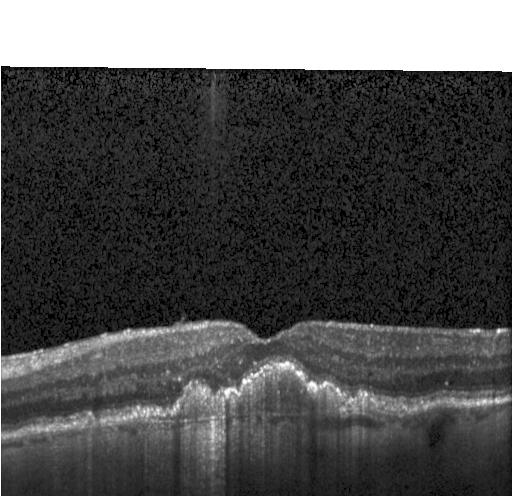 Macular scan. Spectral-domain OCT. OCT line scan
This B-scan demonstrates choroidal neovascularization.